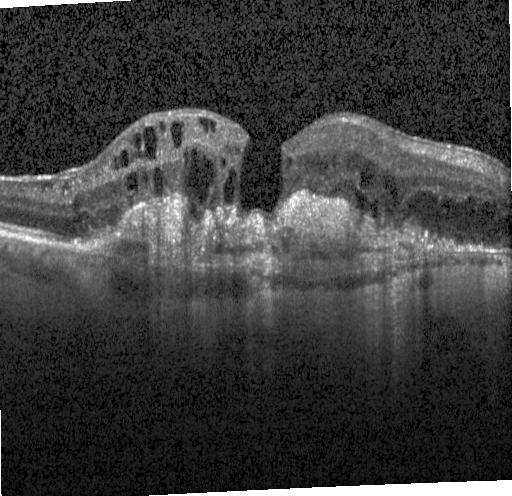
Diagnosis: choroidal neovascularization.